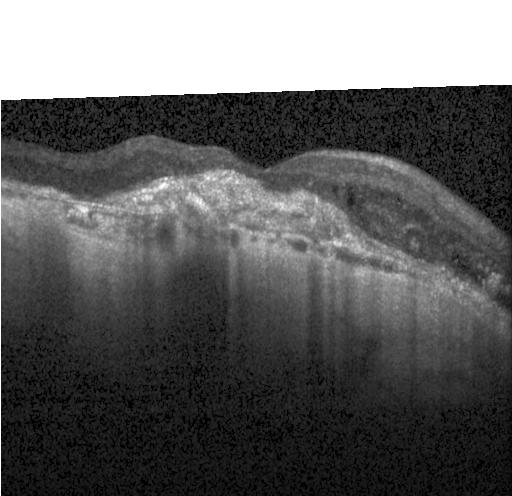 Finding: choroidal neovascularization (CNV).